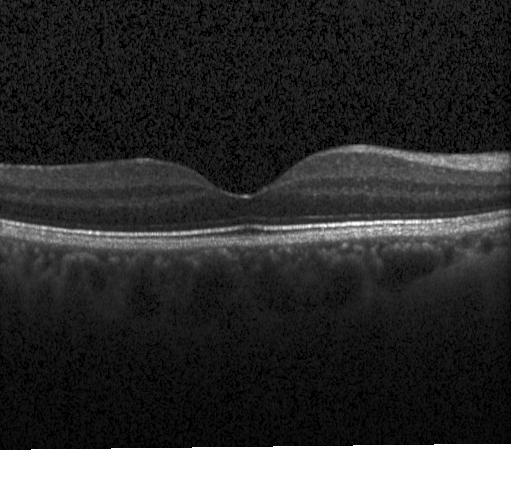 Optical coherence tomography scan · acquired on a Heidelberg Spectralis — The scan shows no choroidal neovascularization, no diabetic macular edema, and no drusen.